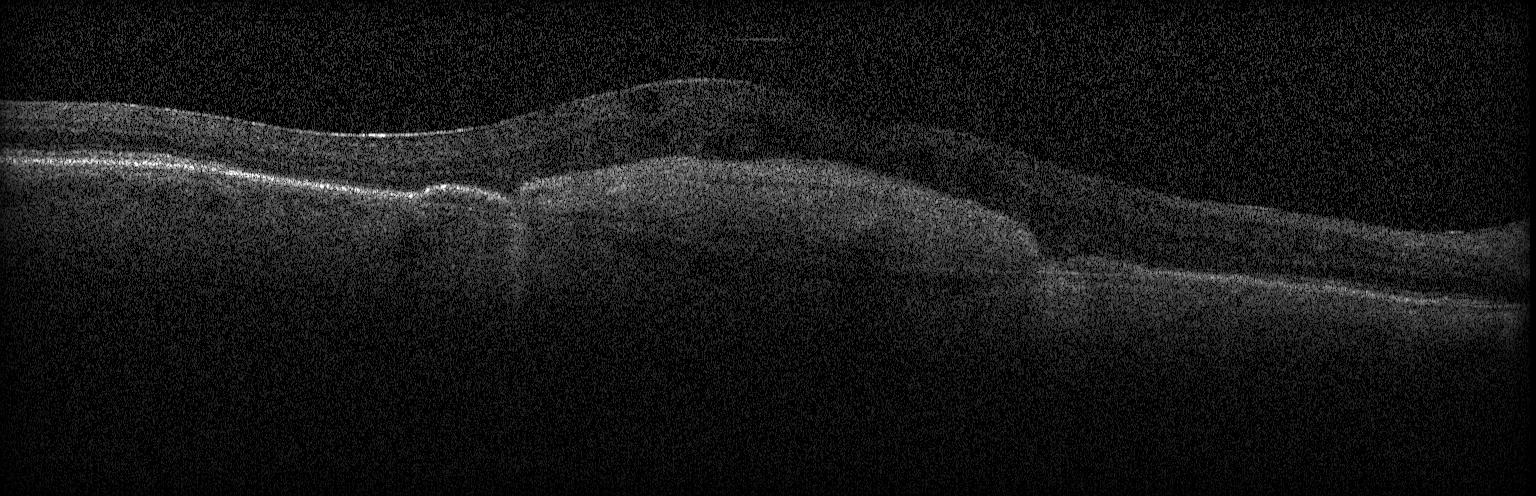
Impression: a choroidal neovascular membrane.